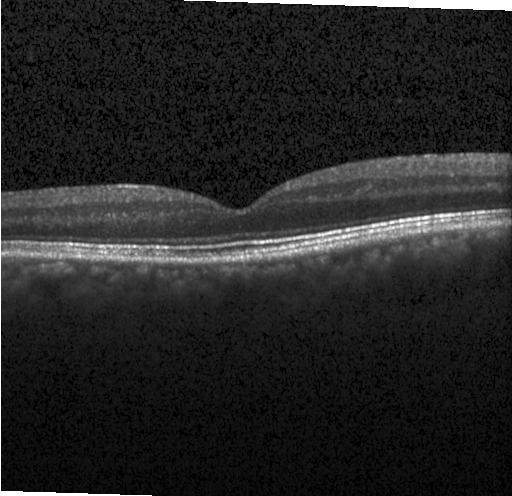

Retinal OCT cross-section. Diagnosis: no choroidal neovascularization, diabetic macular edema, or drusen.